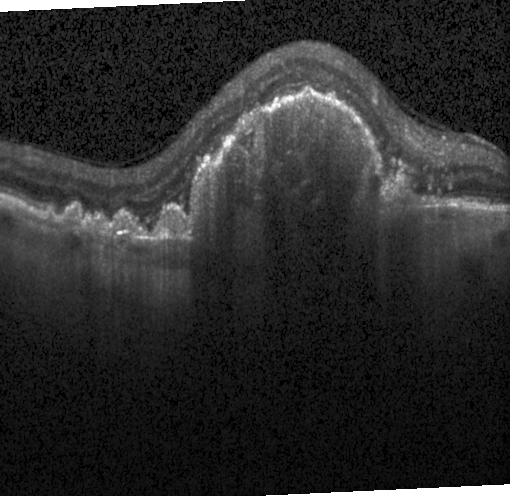 OCT line scan. Spectral-domain optical coherence tomography. Acquired on a Heidelberg Spectralis. Dx: choroidal neovascularization (CNV).